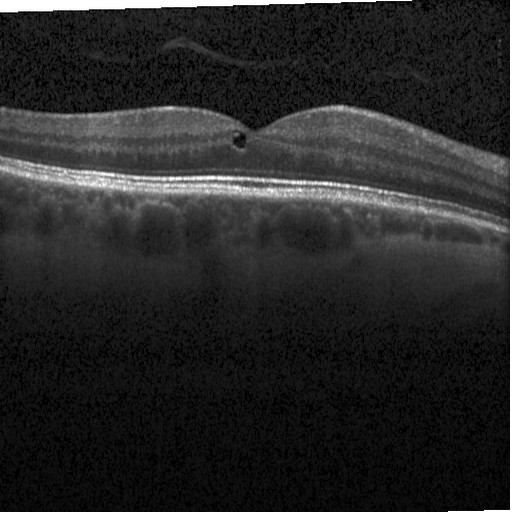 Instrument: Heidelberg Spectralis. OCT line scan — Assessment: DME.